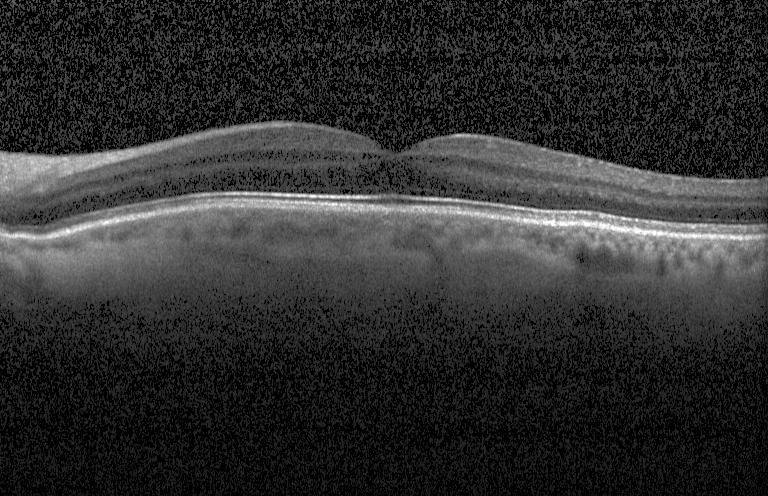 Centered on the fovea, OCT B-scan. Finding: neither choroidal neovascularization, diabetic macular edema, nor drusen.